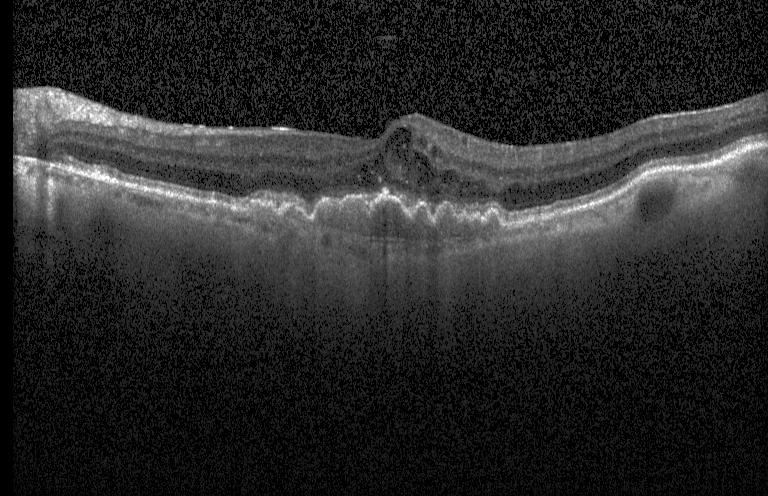
Through the macula · Heidelberg Spectralis OCT system · optical coherence tomography B-scan · SD-OCT. This B-scan demonstrates a choroidal neovascular membrane.